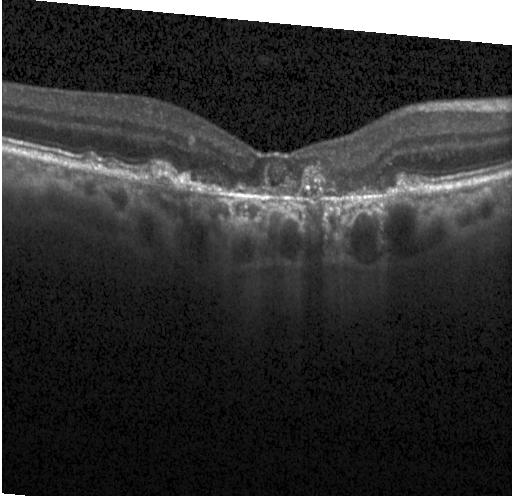

Instrument: Heidelberg Spectralis, SD-OCT, OCT line scan
CNV.